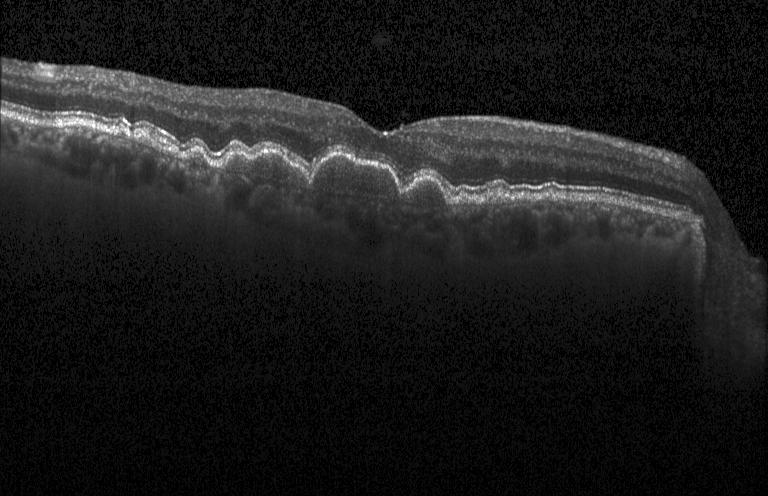
Spectral-domain OCT · centered on the fovea · Heidelberg Spectralis · OCT B-scan — OCT finding: drusen.